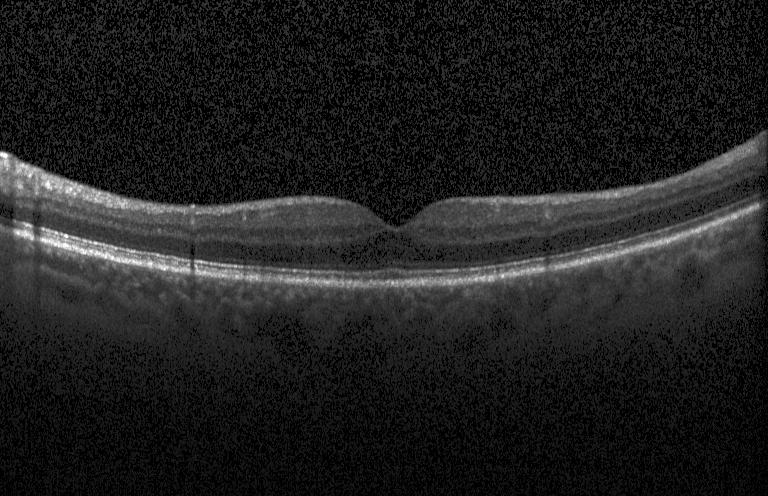

Spectral-domain optical coherence tomography; OCT B-scan. Macular OCT: no CNV, no DME, and no drusen.